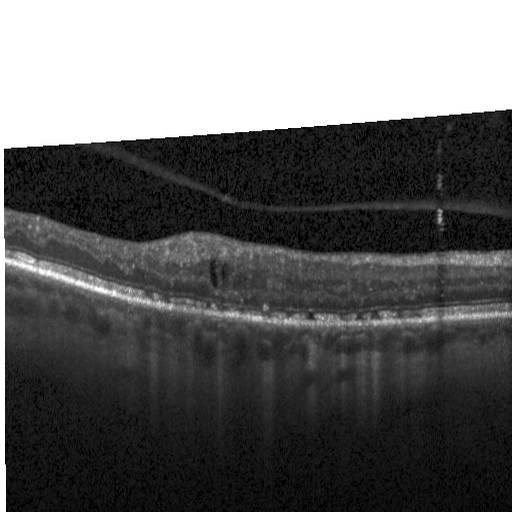

This B-scan demonstrates DME.